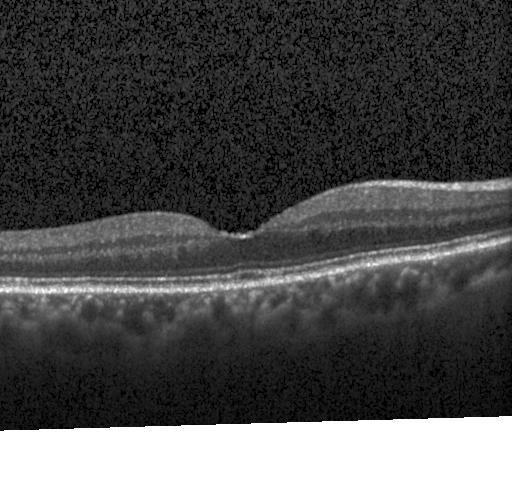 Optical coherence tomography scan. Macular scan. Spectral-domain OCT. Instrument: Heidelberg Spectralis — This B-scan demonstrates neither choroidal neovascularization, diabetic macular edema, nor drusen.